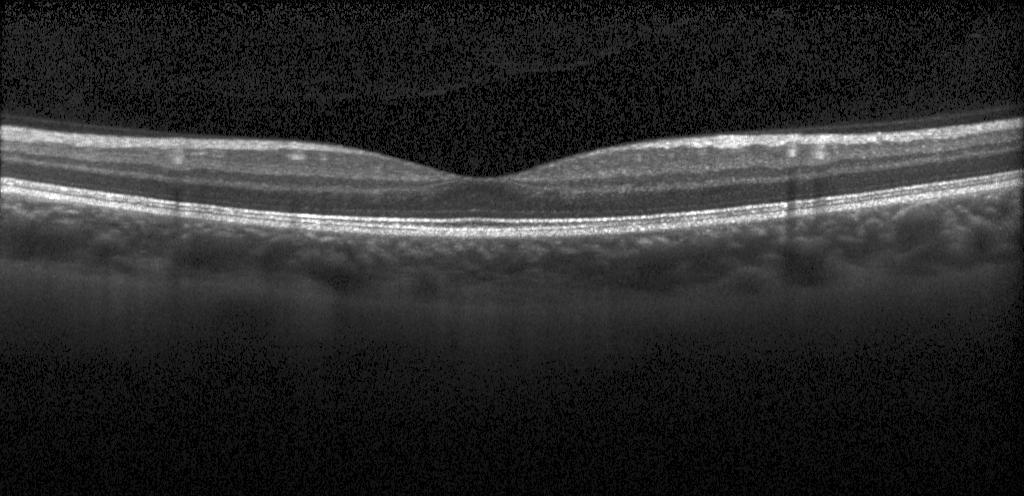

Spectral-domain optical coherence tomography; instrument: Heidelberg Spectralis; OCT B-scan — The scan shows no choroidal neovascularization, diabetic macular edema, or drusen.